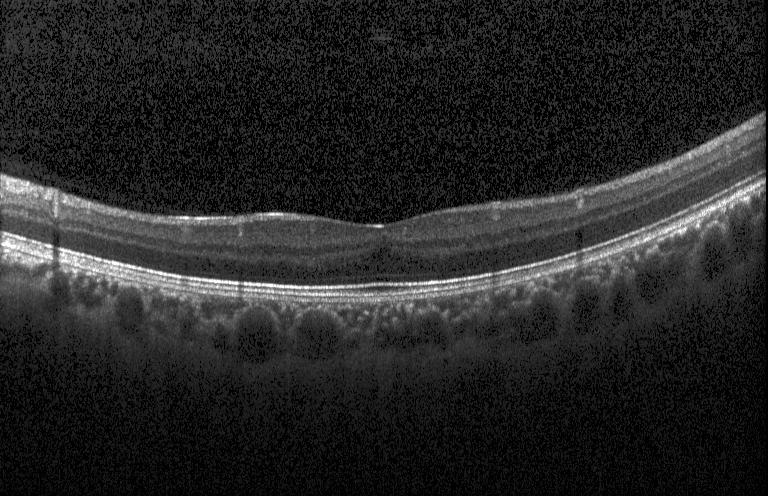

Impression: no evidence of choroidal neovascularization, diabetic macular edema, or drusen.